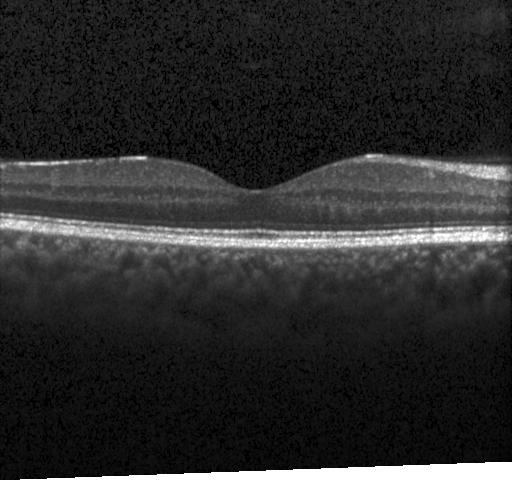

SD-OCT · Heidelberg Spectralis OCT system · retinal OCT cross-section — Impression: no CNV, no DME, and no drusen.